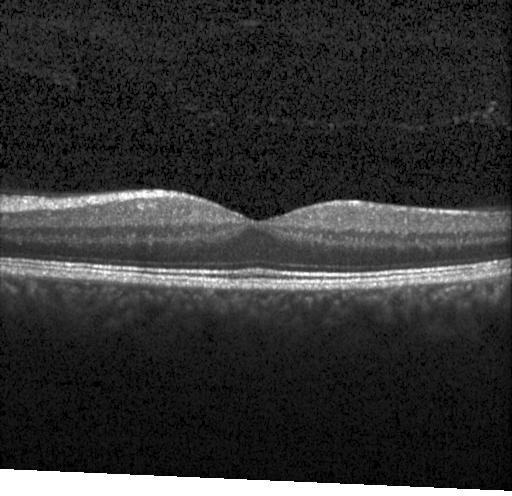

Optical coherence tomography scan
Macular OCT: no CNV, no DME, and no drusen.